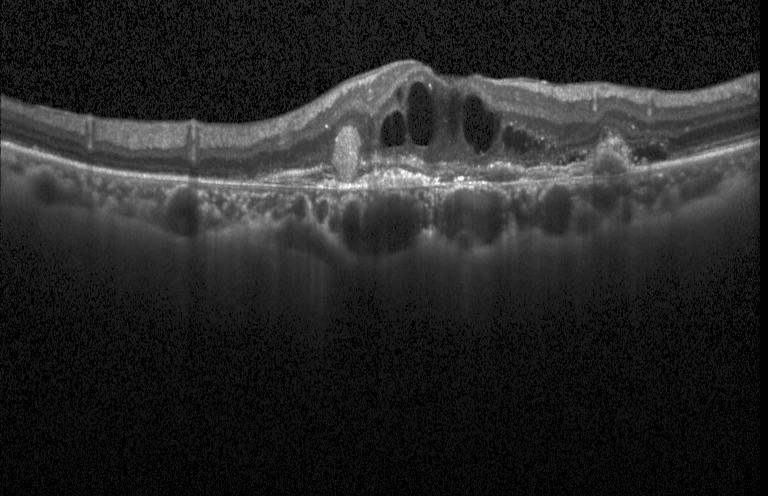 Impression: a choroidal neovascular membrane.